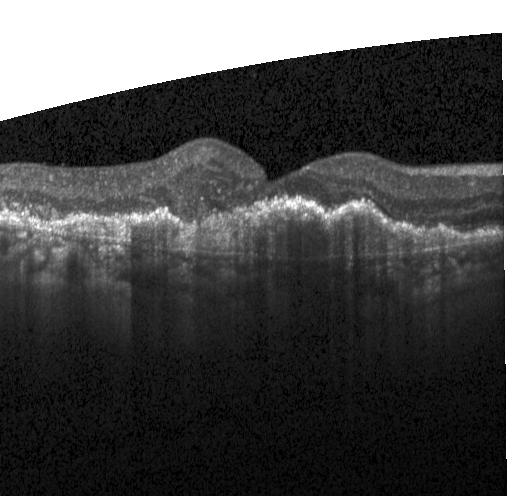

OCT scan showing a choroidal neovascular membrane.